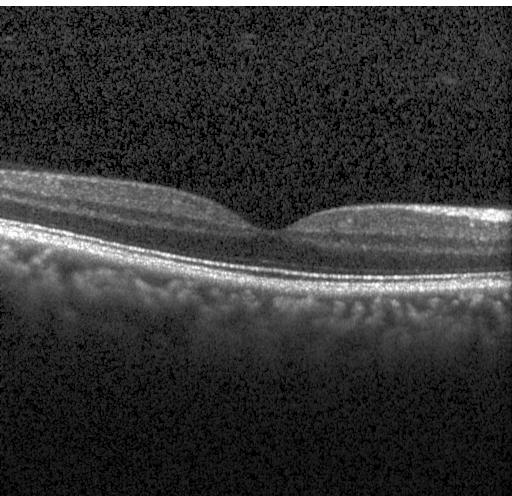 Heidelberg Spectralis; centered on the fovea; OCT B-scan — Impression: neither CNV, DME, nor drusen.